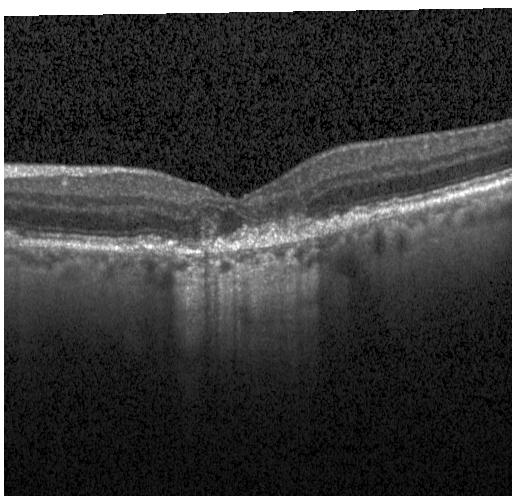
Dx: a choroidal neovascular membrane.